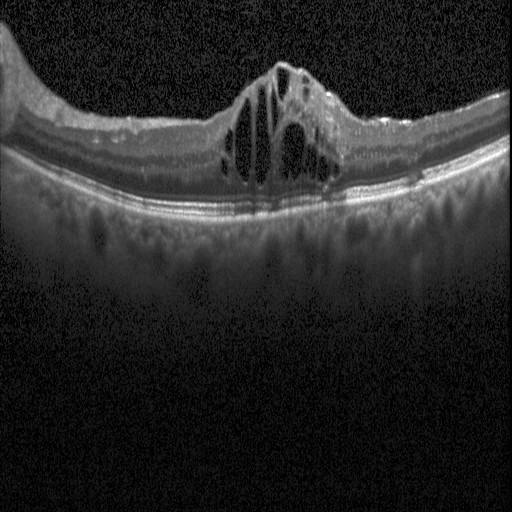

Macular scan. Spectral-domain optical coherence tomography. Heidelberg Spectralis OCT system. Optical coherence tomography B-scan — Finding: diabetic macular edema (DME).